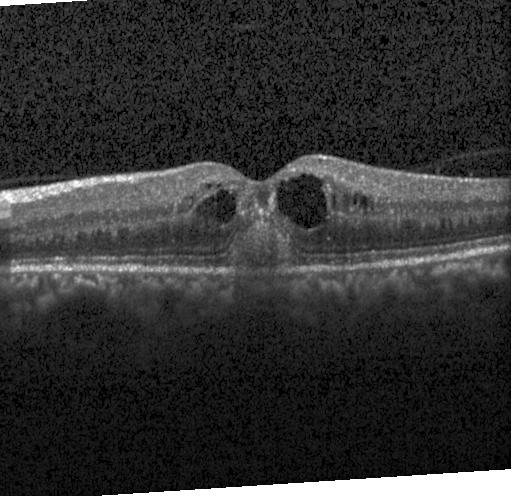
OCT scan showing CNV.